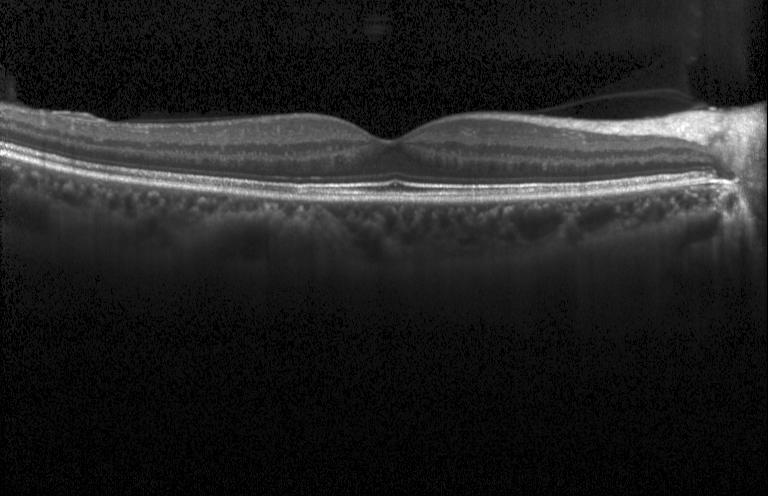 Spectral-domain OCT. Retinal OCT cross-section.
Dx: neither CNV, DME, nor drusen.